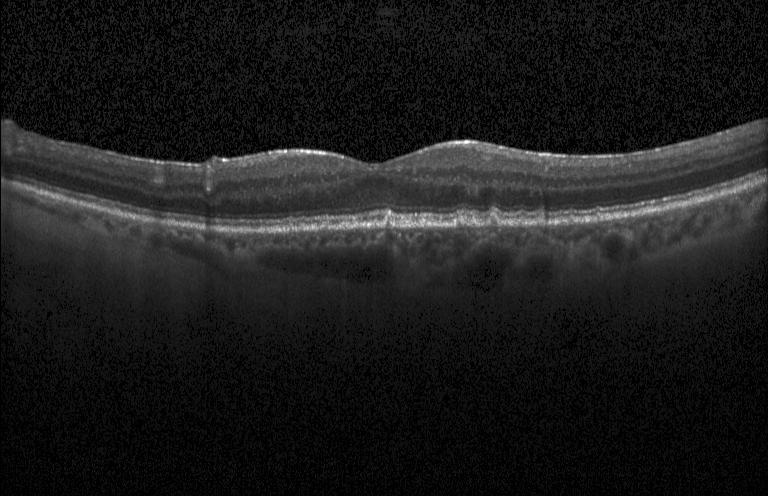 Finding: multiple drusen.